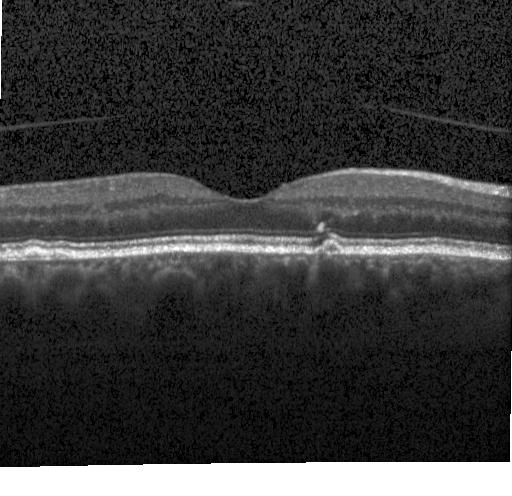

Heidelberg Spectralis, spectral-domain OCT, OCT line scan
Dx: sub-RPE drusenoid deposits.